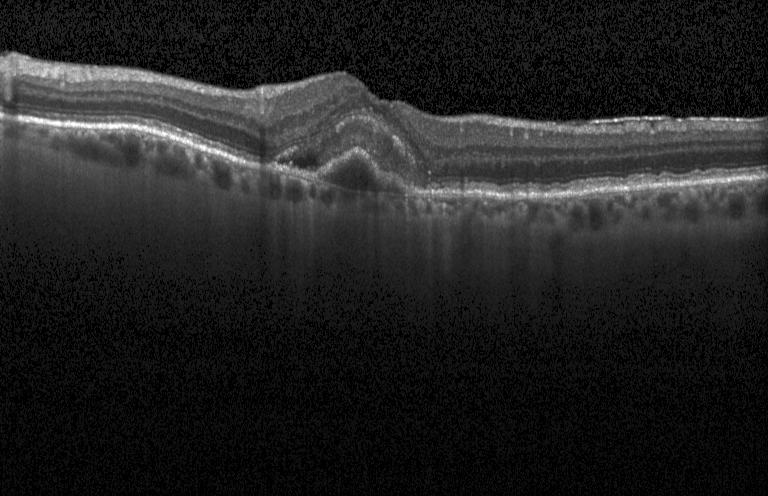 Finding: CNV.